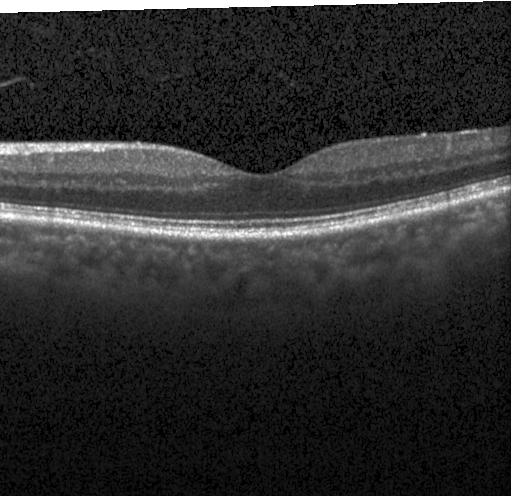 Acquired on a Heidelberg Spectralis, spectral-domain OCT, retinal OCT B-scan
Impression: neither choroidal neovascularization, diabetic macular edema, nor drusen.